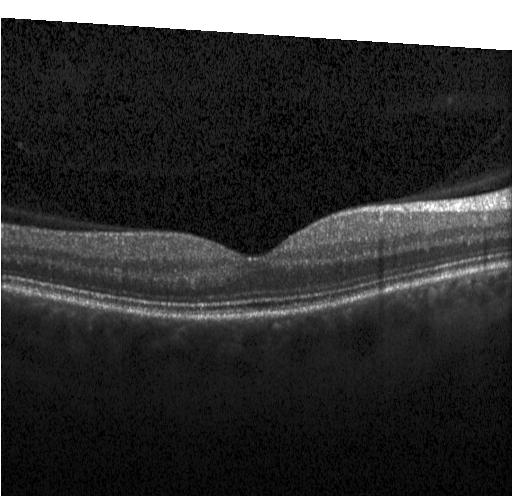

Retinal OCT cross-section
Assessment: no choroidal neovascularization, no diabetic macular edema, and no drusen.